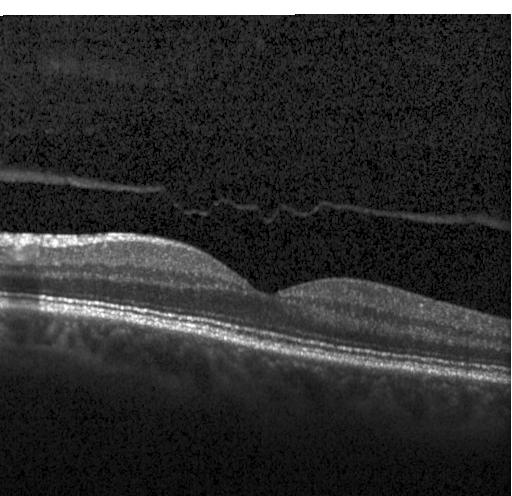 Centered on the fovea. Optical coherence tomography scan — Diagnosis: no CNV, DME, or drusen.